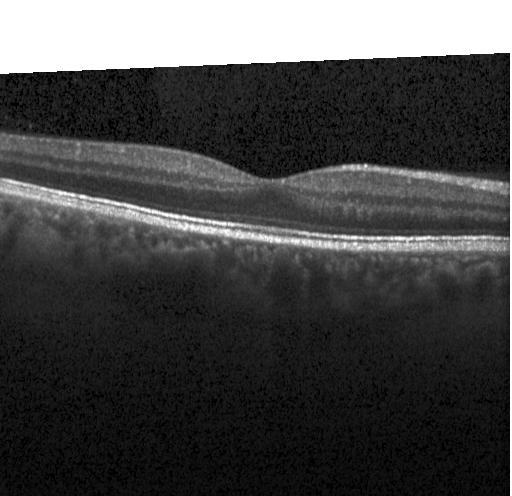
Through the macula. OCT line scan
No evidence of choroidal neovascularization, diabetic macular edema, or drusen.